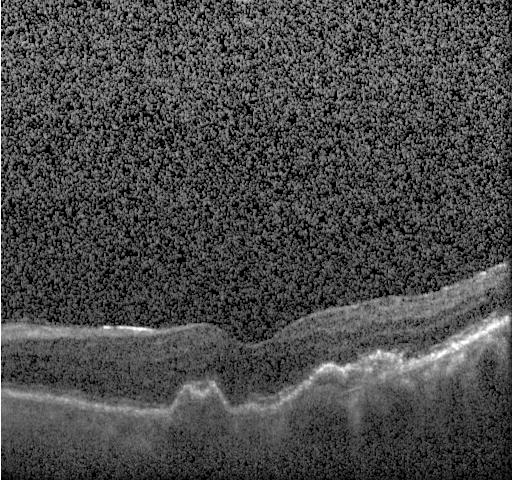 Horizontal scan through the fovea · Heidelberg Spectralis · OCT B-scan · spectral-domain optical coherence tomography
The scan shows a choroidal neovascular membrane.